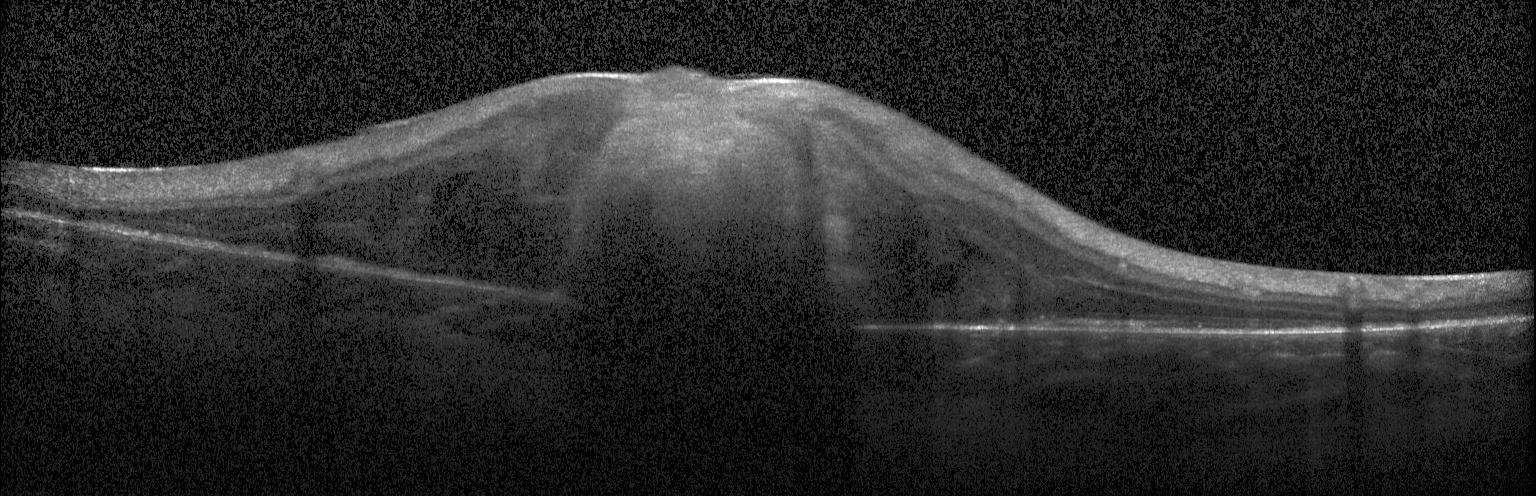 OCT B-scan · centered on the fovea.
CNV.